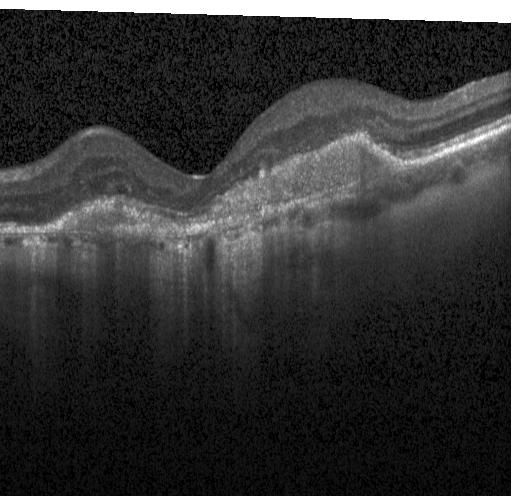 Through the macula, optical coherence tomography B-scan, SD-OCT, acquired on a Heidelberg Spectralis
OCT finding: a choroidal neovascular membrane.